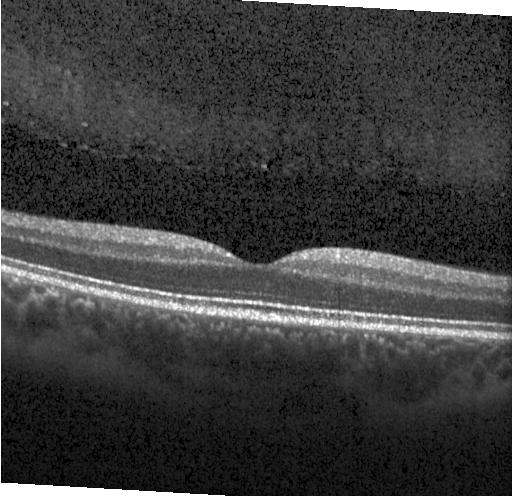 Finding: no evidence of choroidal neovascularization, diabetic macular edema, or drusen.